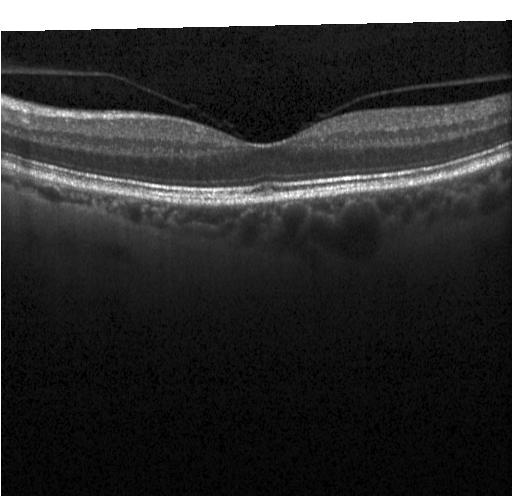
OCT B-scan showing neither choroidal neovascularization, diabetic macular edema, nor drusen.